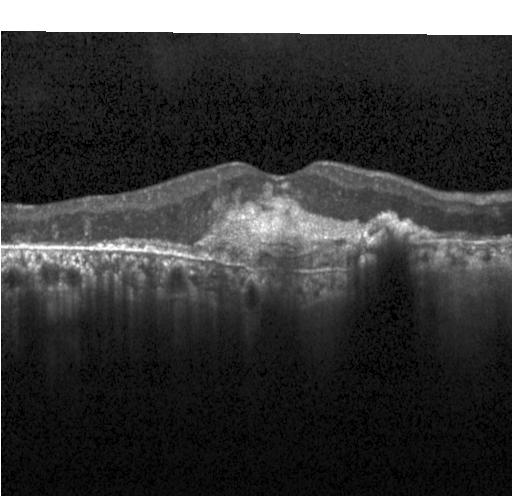 Assessment: a choroidal neovascular membrane.